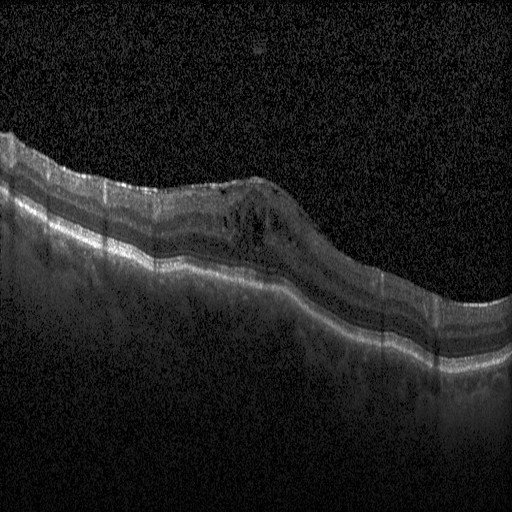

Diagnosis: diabetic macular edema (DME).